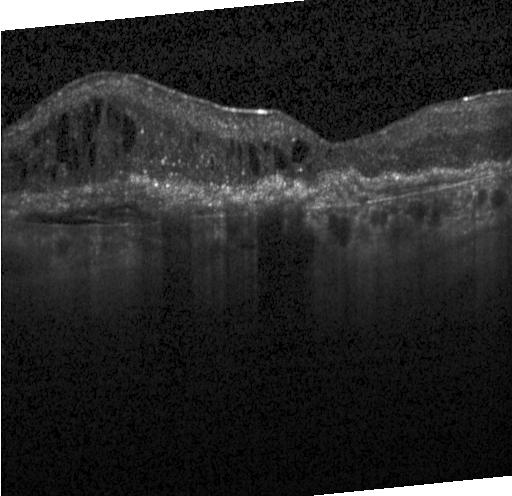
OCT line scan, spectral-domain OCT, acquired on a Heidelberg Spectralis. Finding: a choroidal neovascular membrane.